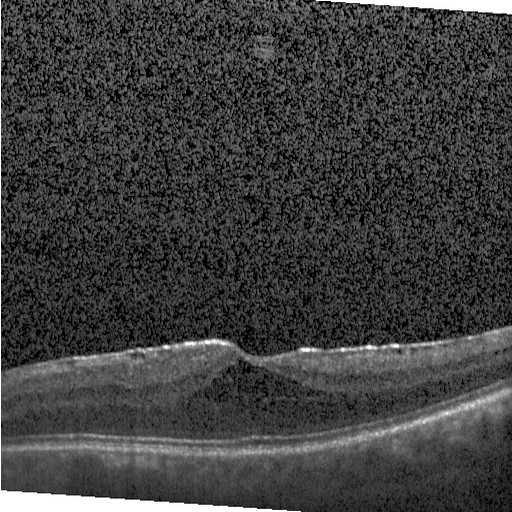 Heidelberg Spectralis · macular scan · spectral-domain optical coherence tomography · optical coherence tomography B-scan.
Dx: DME.